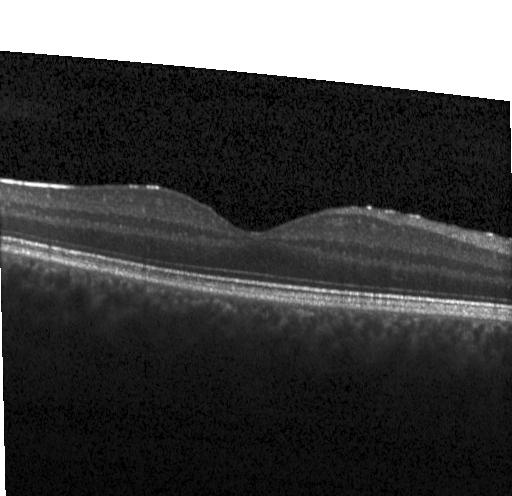 Retinal OCT cross-section. Neither CNV, DME, nor drusen.